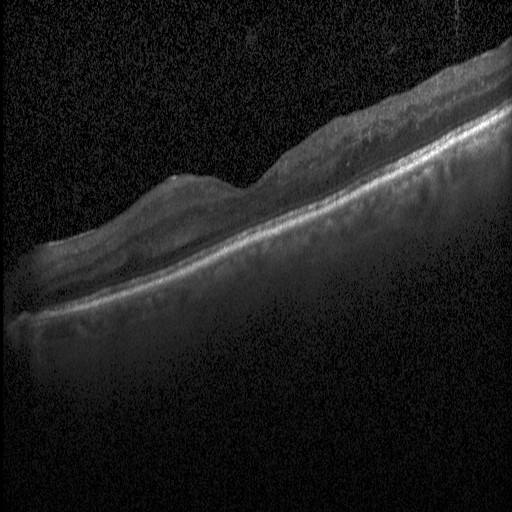

The scan shows diabetic macular edema (DME).